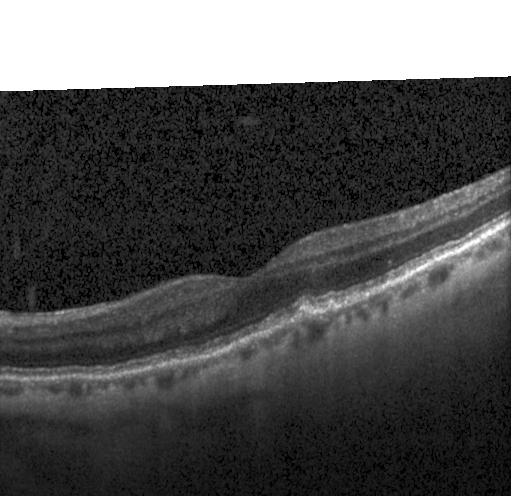
Retinal OCT cross-section
Diagnosis: drusen.